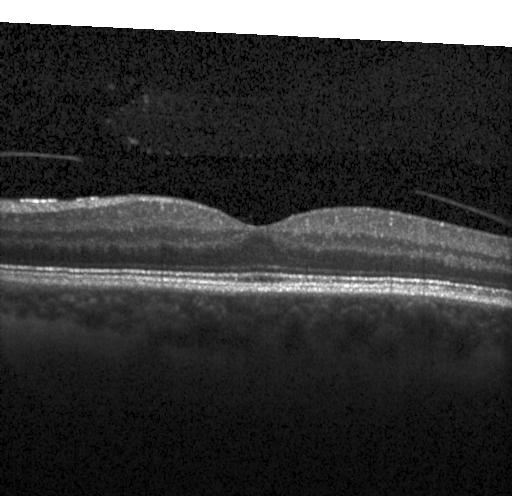 Centered on the fovea; SD-OCT; retinal OCT cross-section; Heidelberg Spectralis OCT system
Dx: no evidence of choroidal neovascularization, diabetic macular edema, or drusen.